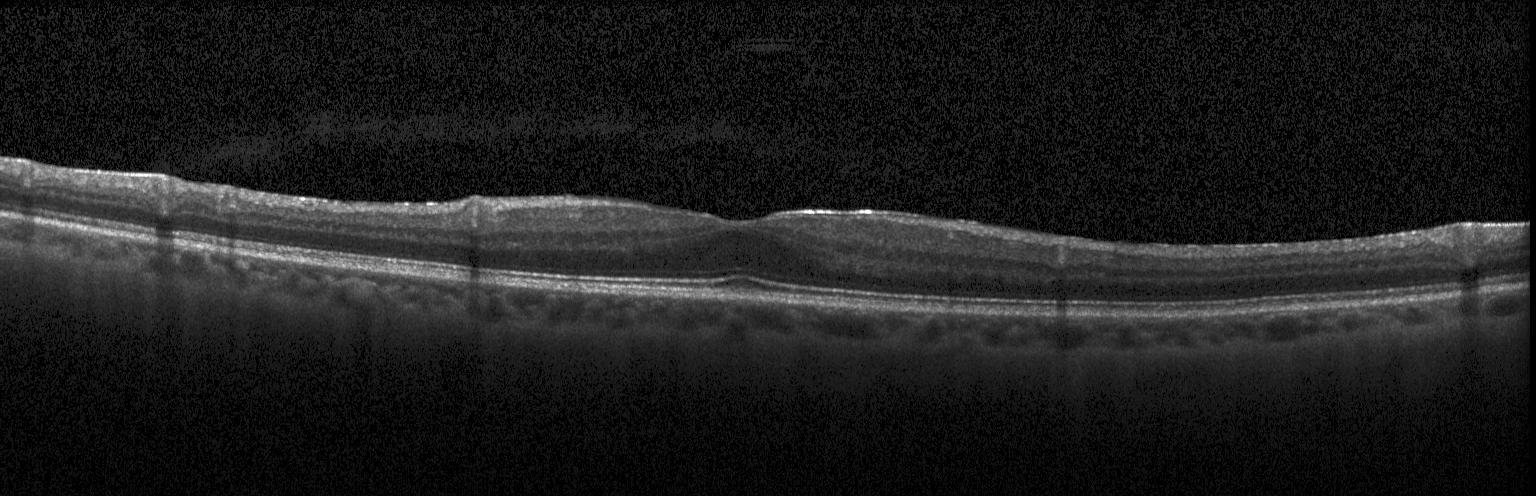
Instrument: Heidelberg Spectralis. OCT line scan — The scan shows no CNV, no DME, and no drusen.